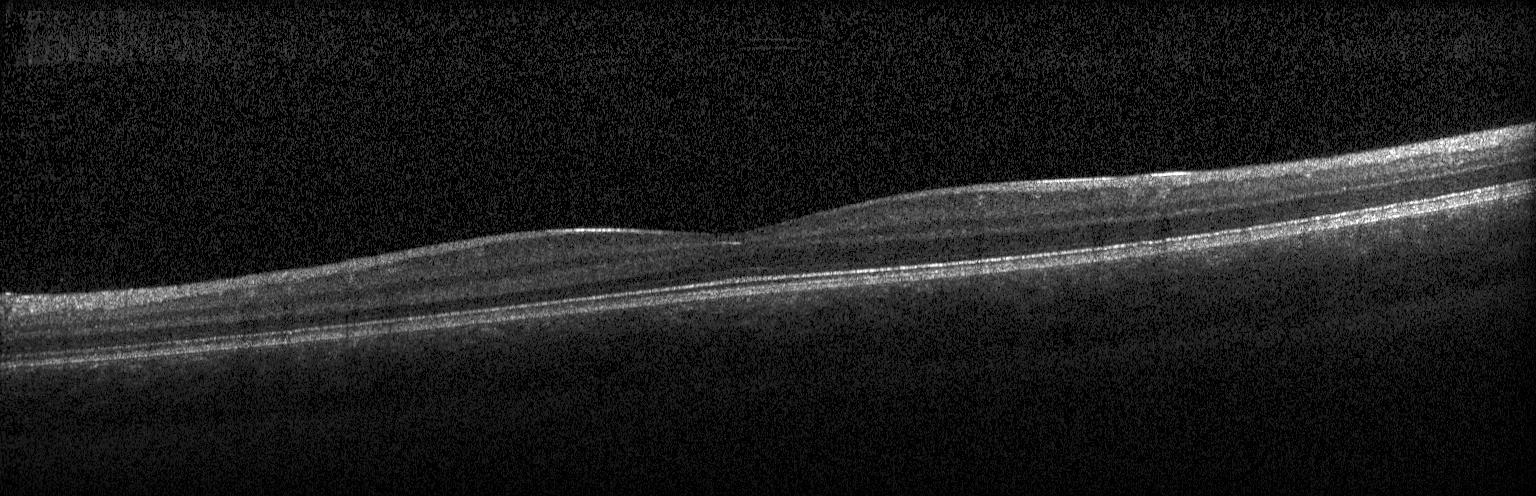 SD-OCT. Acquired on a Heidelberg Spectralis. Retinal OCT B-scan. Macular OCT: no choroidal neovascularization, no diabetic macular edema, and no drusen.